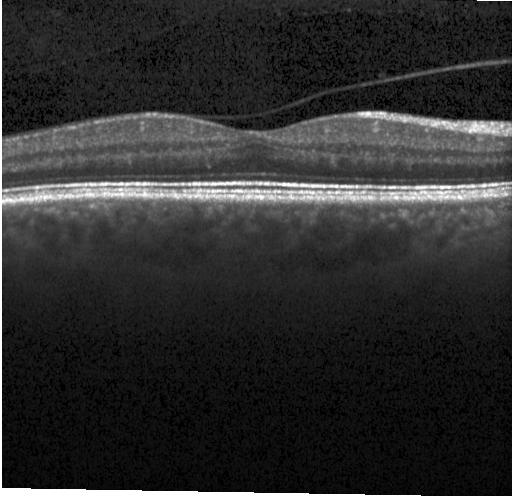
Retinal OCT cross-section · spectral-domain optical coherence tomography.
This B-scan demonstrates neither choroidal neovascularization, diabetic macular edema, nor drusen.